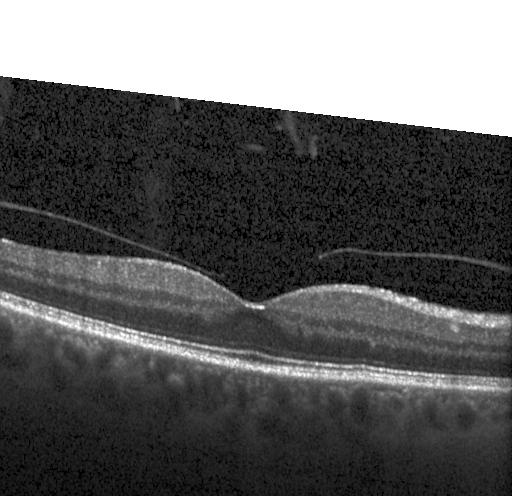
SD-OCT; OCT B-scan — Finding: no evidence of choroidal neovascularization, diabetic macular edema, or drusen.